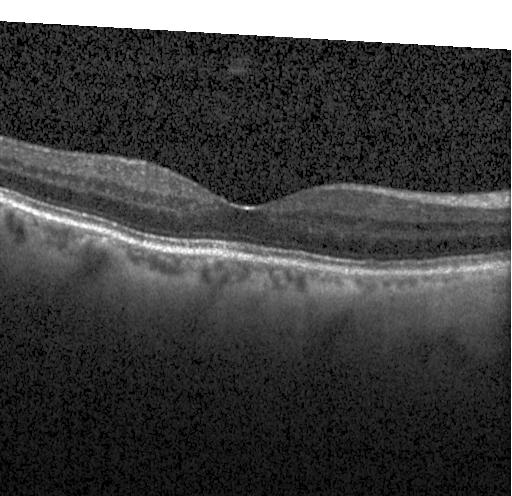
Spectral-domain optical coherence tomography · OCT B-scan
Impression: neither choroidal neovascularization, diabetic macular edema, nor drusen.